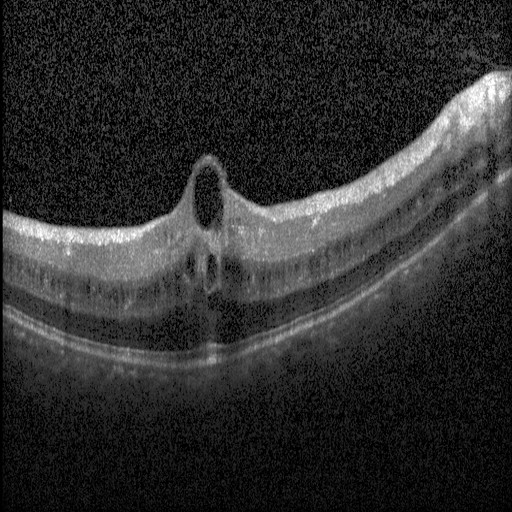 Assessment: DME.